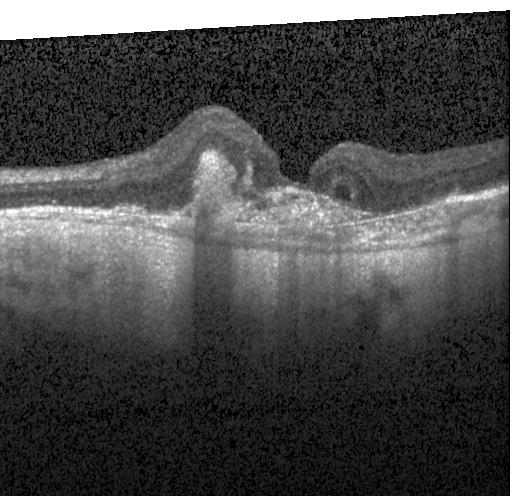
OCT B-scan.
Dx: CNV.